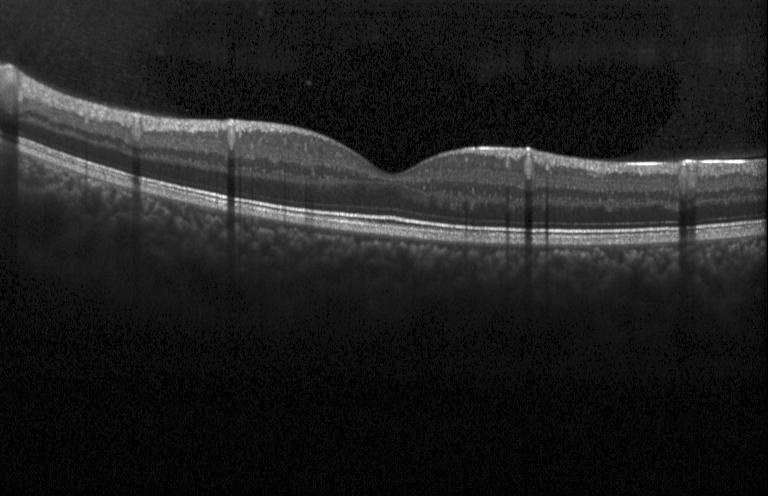

Optical coherence tomography scan. SD-OCT — Assessment: no choroidal neovascularization, no diabetic macular edema, and no drusen.